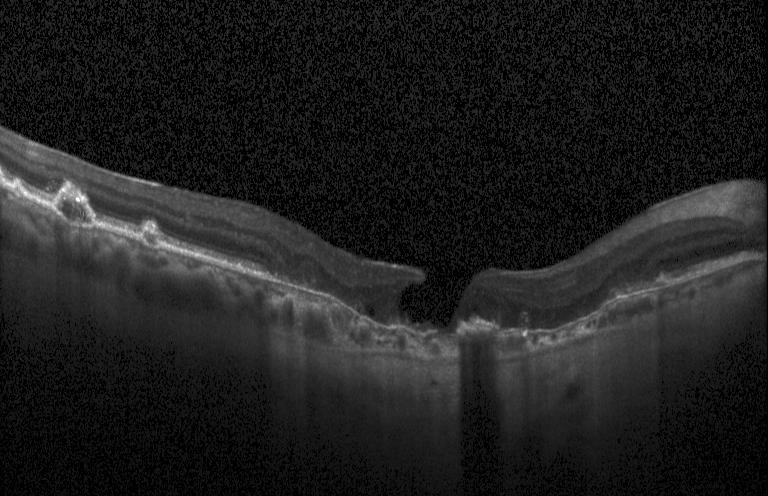
OCT scan showing choroidal neovascularization.